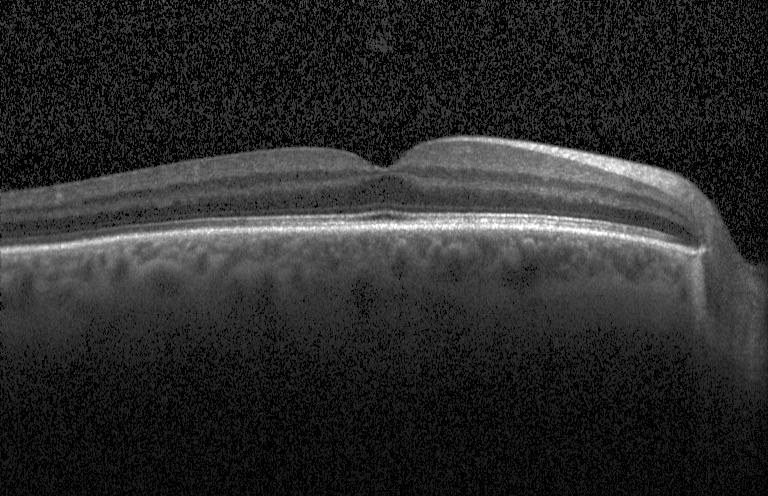 OCT B-scan — This B-scan demonstrates neither choroidal neovascularization, diabetic macular edema, nor drusen.